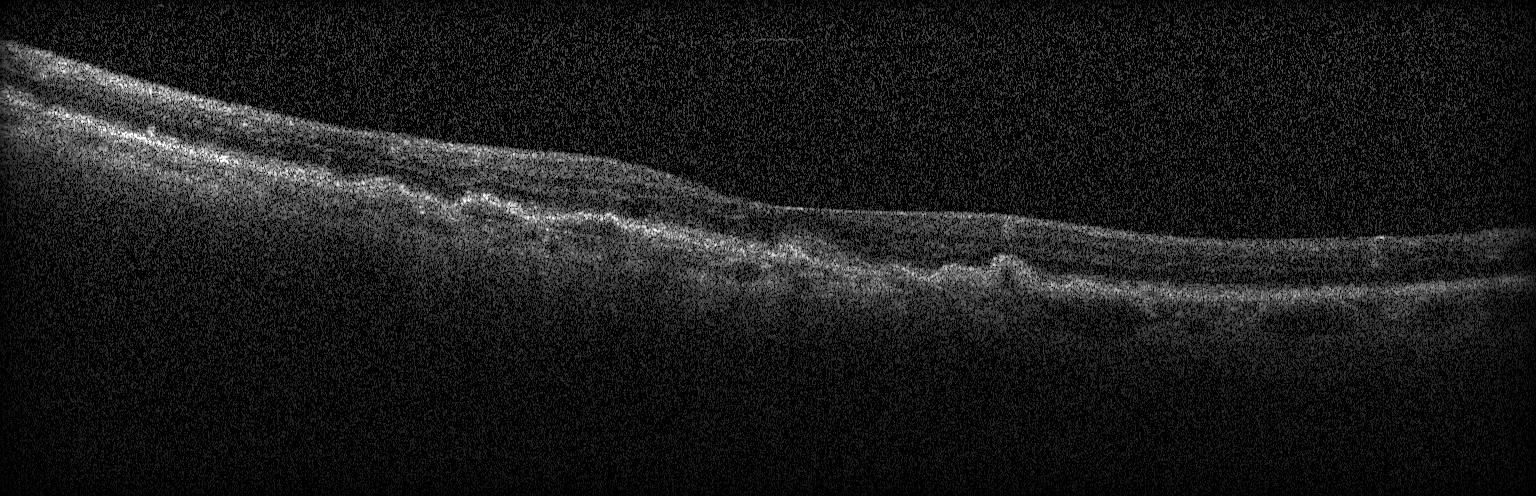 Optical coherence tomography B-scan. This B-scan demonstrates a choroidal neovascular membrane.